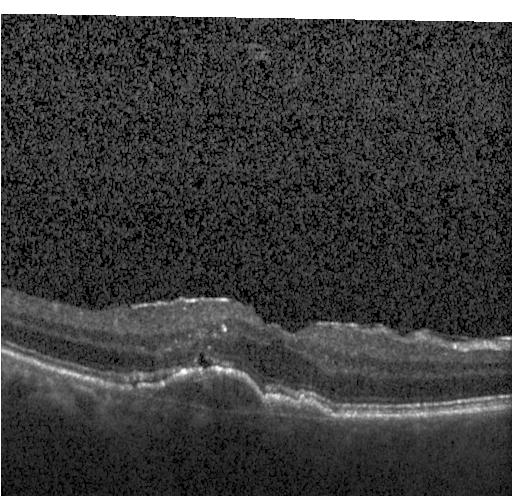 Heidelberg Spectralis · optical coherence tomography B-scan · horizontal scan through the fovea.
Macular OCT: choroidal neovascularization (CNV).